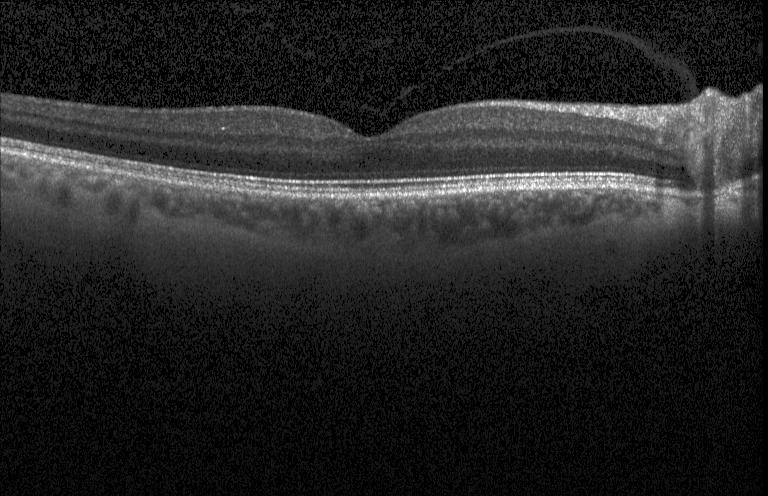
Heidelberg Spectralis OCT system. Retinal OCT B-scan. Assessment: no choroidal neovascularization, no diabetic macular edema, and no drusen.